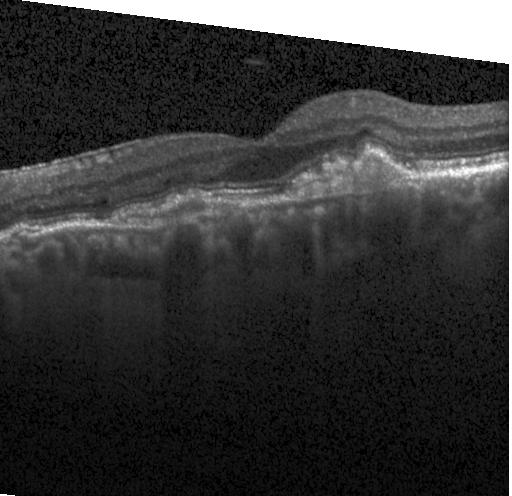

Finding: a choroidal neovascular membrane.